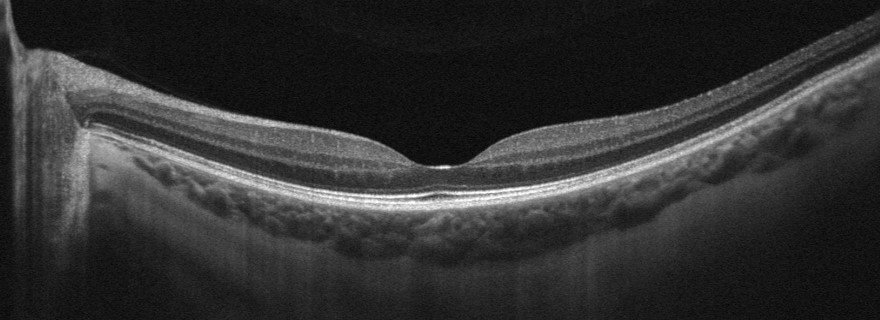 OCT scan showing no AMD, DME, ERM, RAO, RVO, or VID.